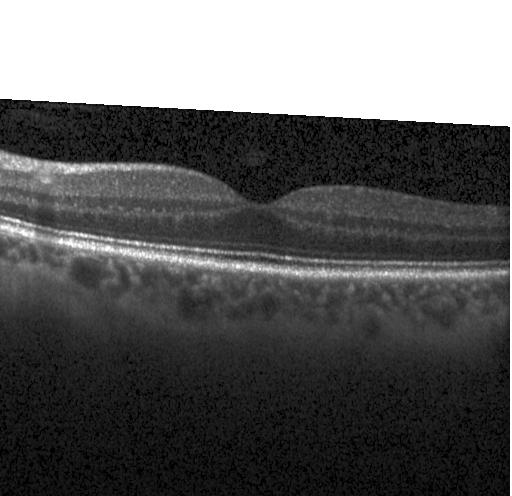

Spectral-domain OCT; retinal OCT B-scan; acquired on a Heidelberg Spectralis — This B-scan demonstrates no evidence of CNV, DME, or drusen.